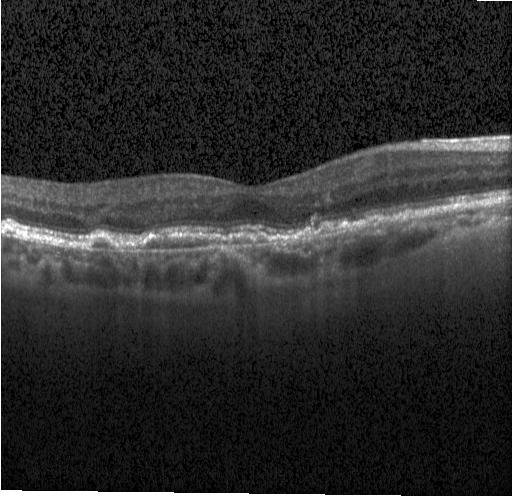 Macular scan; OCT line scan
Impression: a choroidal neovascular membrane.